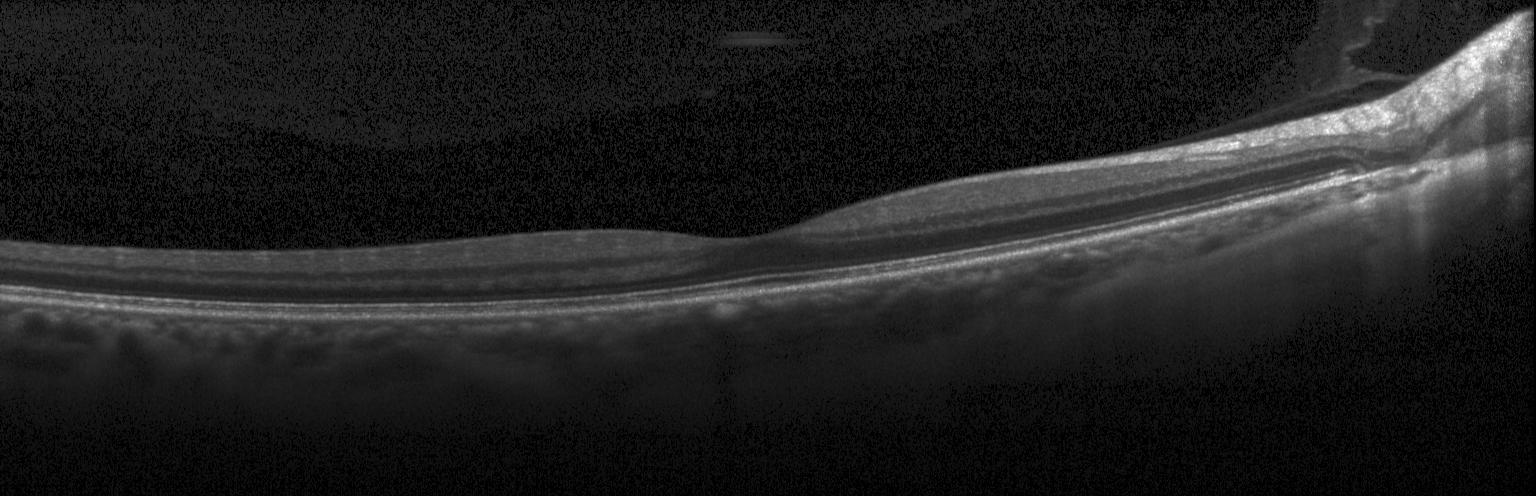

Retinal OCT B-scan · macular scan. Assessment: no choroidal neovascularization, no diabetic macular edema, and no drusen.